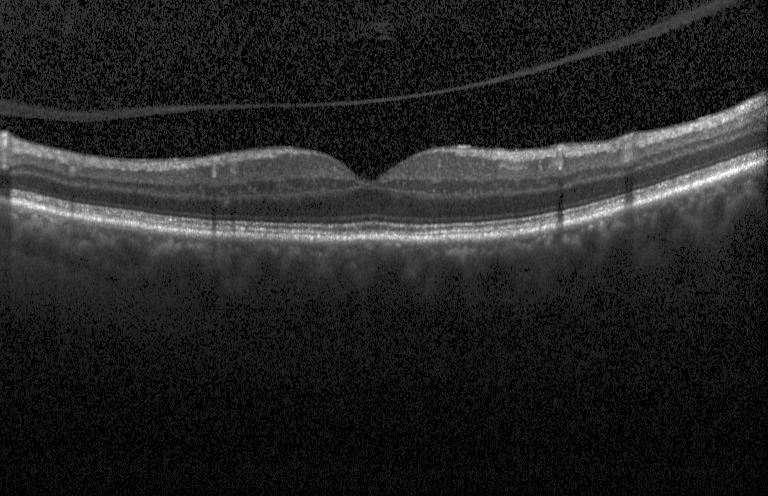 Instrument: Heidelberg Spectralis. OCT line scan — Diagnosis: no choroidal neovascularization, diabetic macular edema, or drusen.